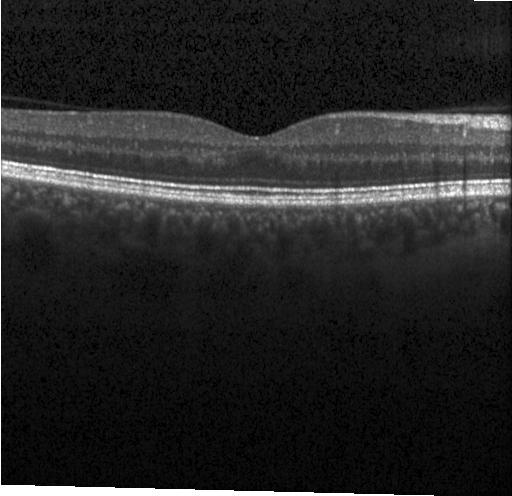

Retinal OCT B-scan, spectral-domain optical coherence tomography, through the macula, Heidelberg Spectralis OCT system.
This B-scan demonstrates no evidence of choroidal neovascularization, diabetic macular edema, or drusen.